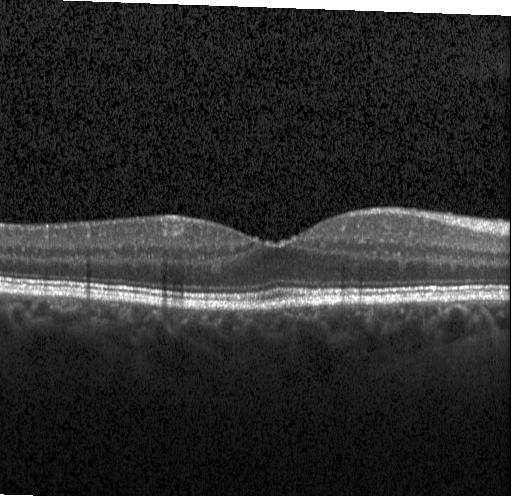
Optical coherence tomography scan · fovea-centered. Impression: no CNV, no DME, and no drusen.